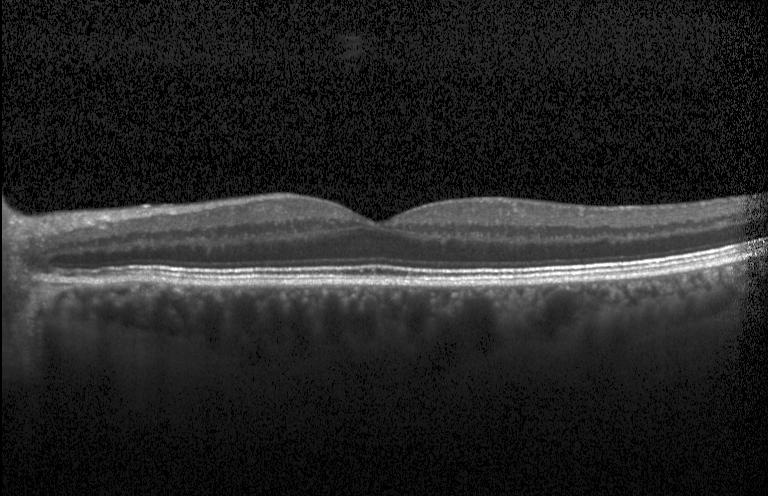

Retinal OCT cross-section. Diagnosis: neither choroidal neovascularization, diabetic macular edema, nor drusen.